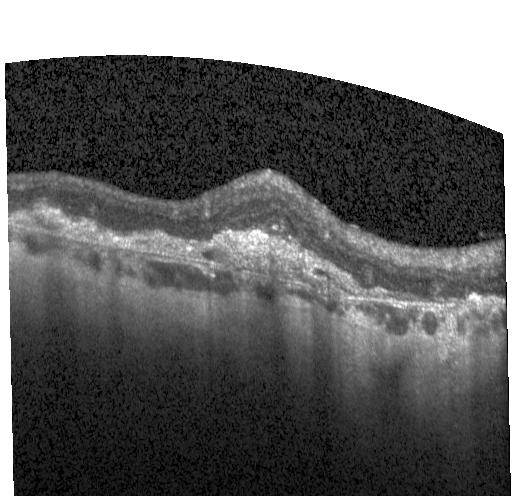
Optical coherence tomography B-scan · centered on the fovea · Heidelberg Spectralis.
Diagnosis: choroidal neovascularization (CNV).